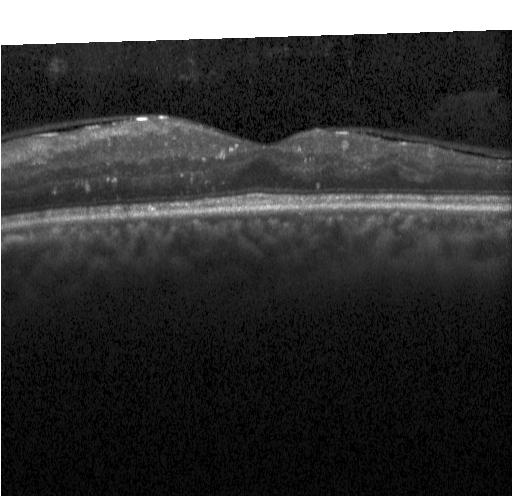

Heidelberg Spectralis OCT system; retinal OCT B-scan; spectral-domain OCT; horizontal scan through the fovea.
Diagnosis: diabetic macular edema (DME).